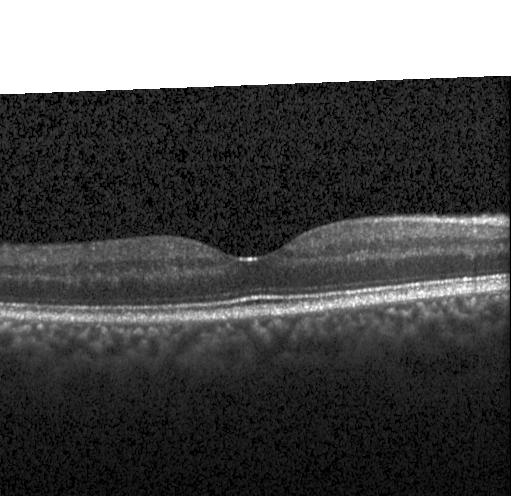 SD-OCT; Heidelberg Spectralis; fovea-centered; optical coherence tomography scan — Finding: no evidence of choroidal neovascularization, diabetic macular edema, or drusen.